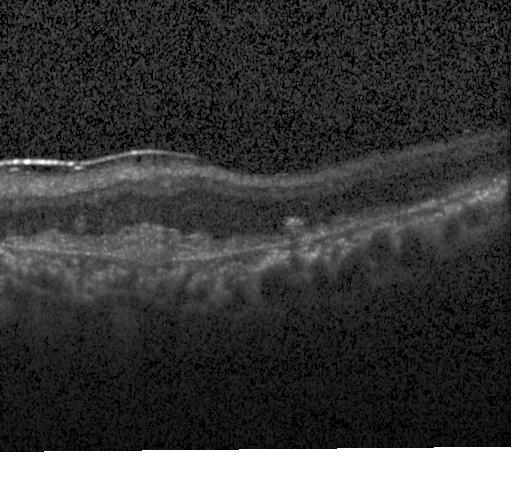 Finding: a choroidal neovascular membrane.